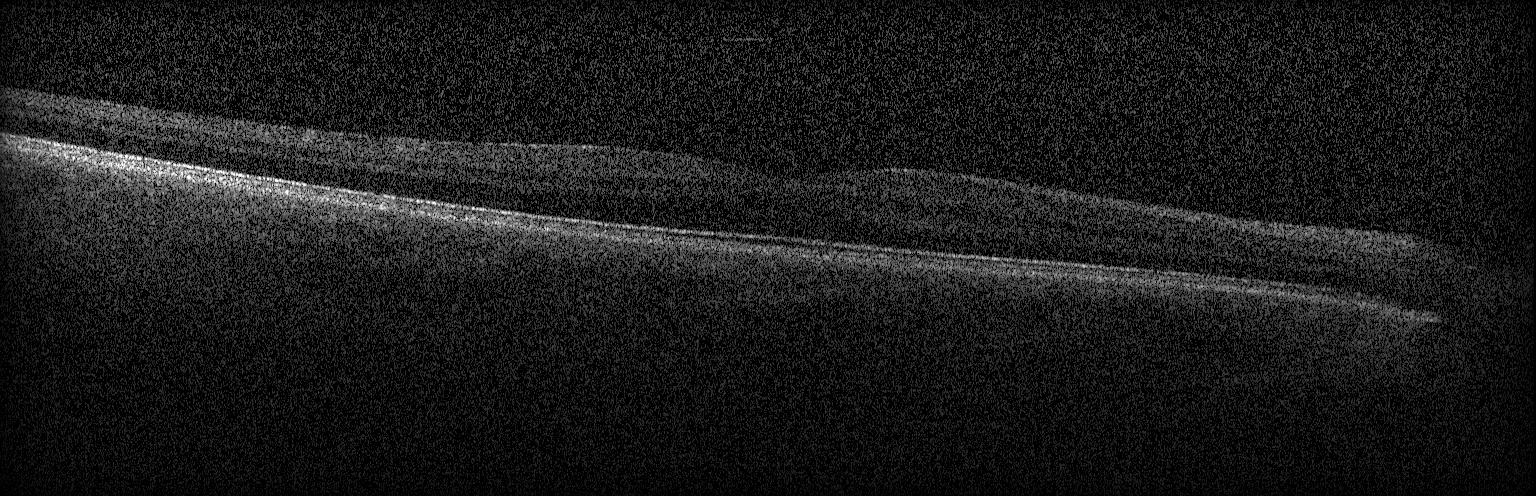

Horizontal scan through the fovea · retinal OCT B-scan
Finding: neither CNV, DME, nor drusen.